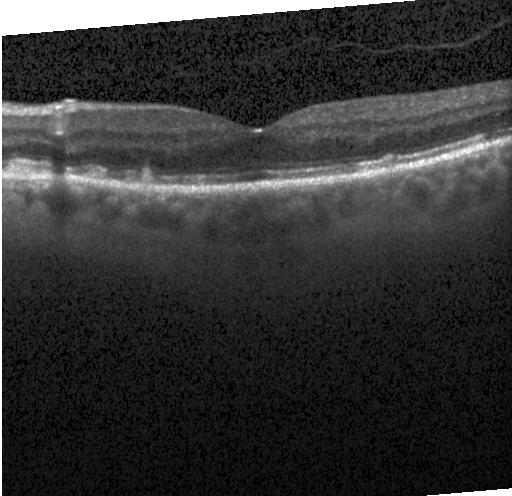

Spectral-domain OCT B-scan: sub-RPE drusenoid deposits.